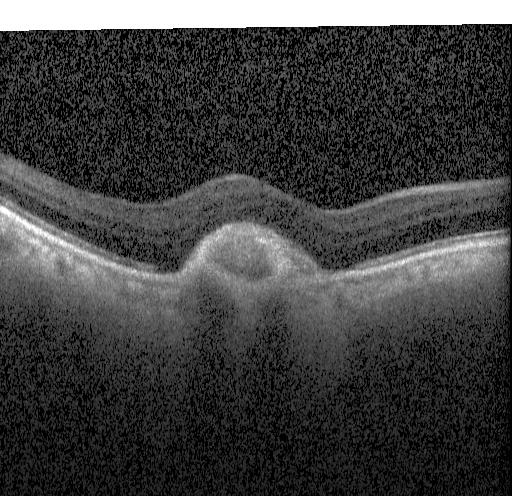

This B-scan demonstrates choroidal neovascularization.